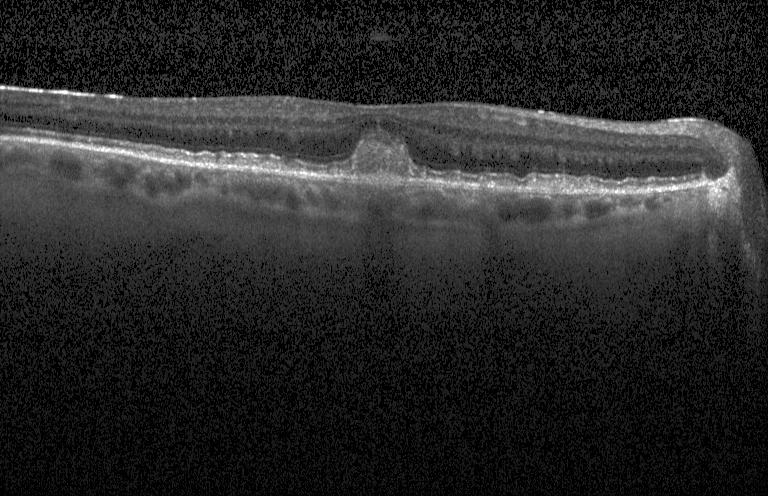
Spectral-domain OCT. OCT line scan. Heidelberg Spectralis. Dx: a choroidal neovascular membrane.